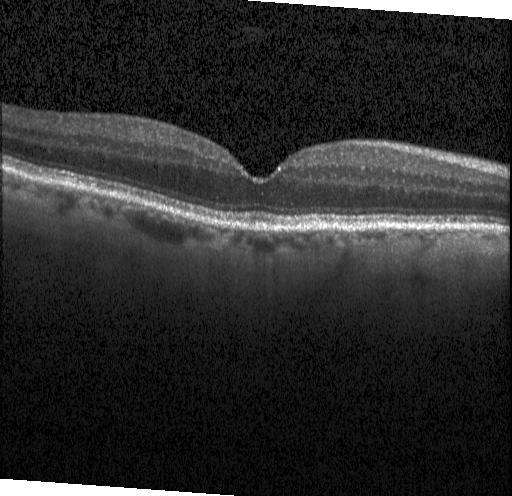

Heidelberg Spectralis. Fovea-centered. OCT line scan. Spectral-domain optical coherence tomography — Finding: no evidence of choroidal neovascularization, diabetic macular edema, or drusen.